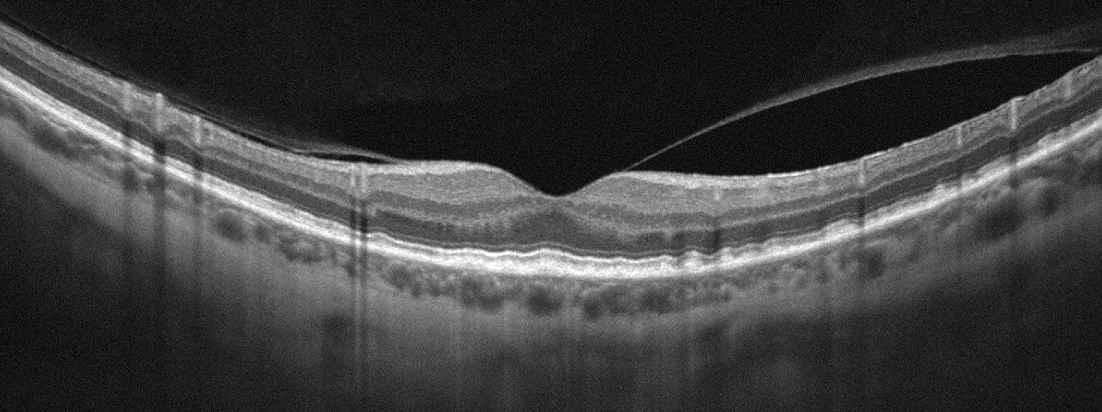 Optovue Avanti RTVue XR; OCT B-scan; through the macula
Dx: age-related macular degeneration.